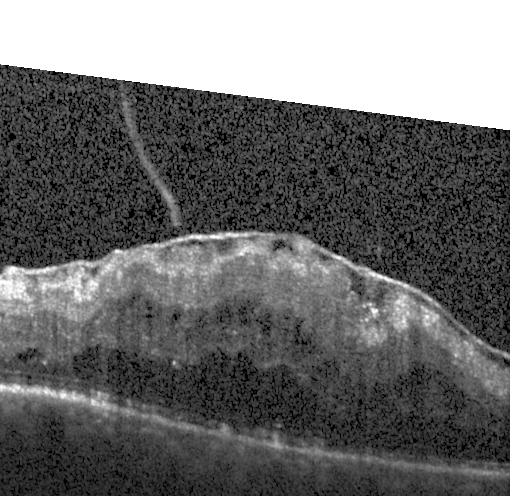

Spectral-domain OCT B-scan: diabetic macular edema.